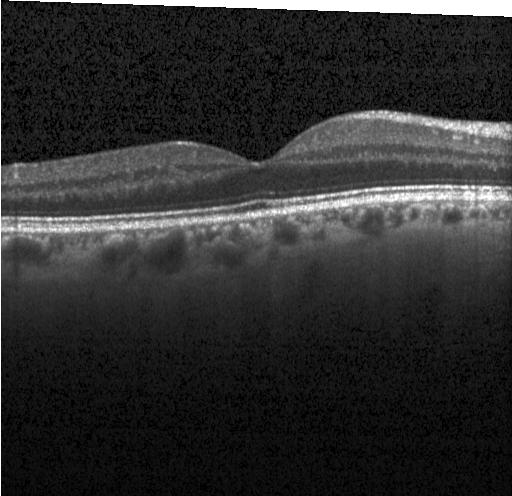
Retinal OCT B-scan · through the macula
This B-scan demonstrates no CNV, DME, or drusen.